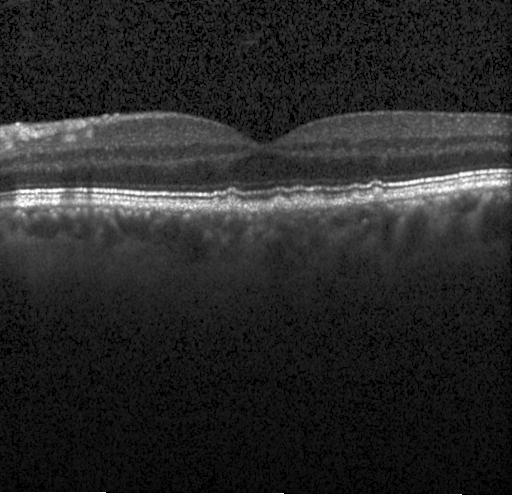
Impression: sub-RPE drusenoid deposits.